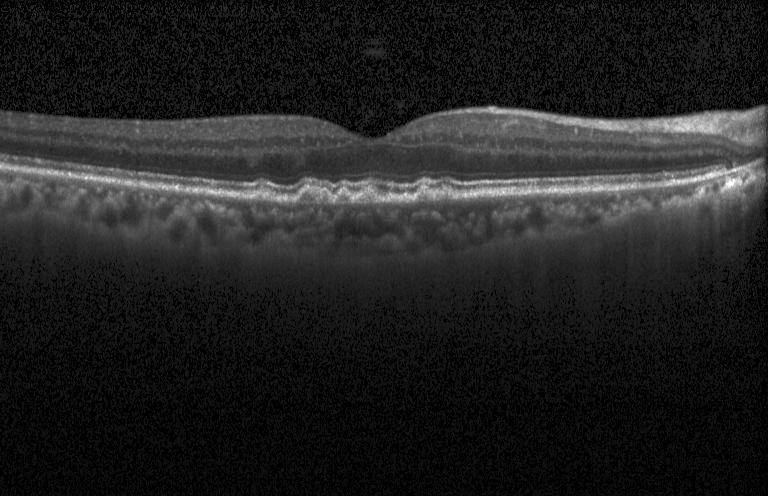

The scan shows drusen.